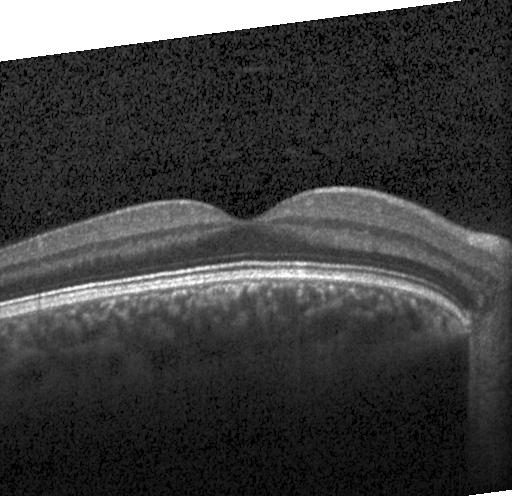 Retinal OCT B-scan.
Diagnosis: no choroidal neovascularization, diabetic macular edema, or drusen.